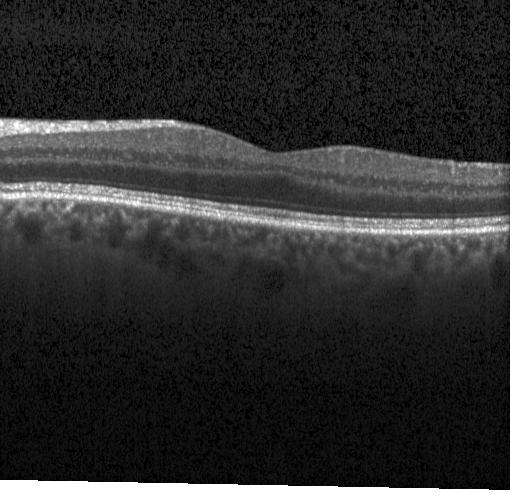
SD-OCT. Centered on the fovea. Optical coherence tomography B-scan.
Impression: no choroidal neovascularization, diabetic macular edema, or drusen.